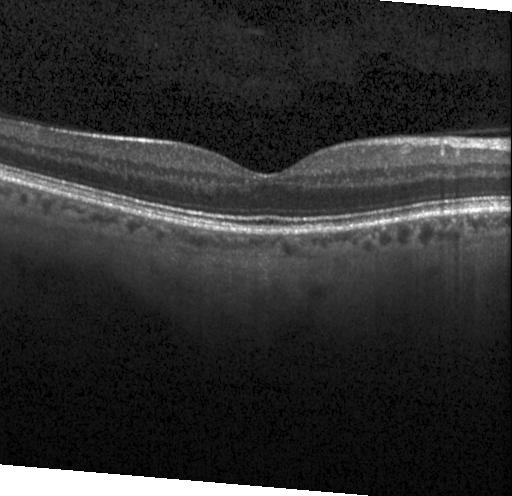

Finding: no choroidal neovascularization, no diabetic macular edema, and no drusen.